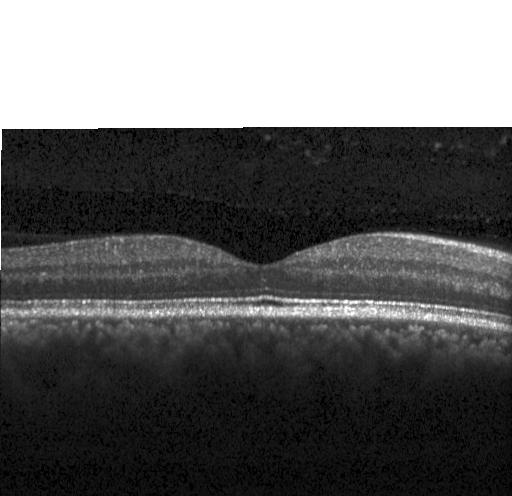 Retinal OCT cross-section · spectral-domain OCT · instrument: Heidelberg Spectralis · through the macula. Assessment: no choroidal neovascularization, no diabetic macular edema, and no drusen.